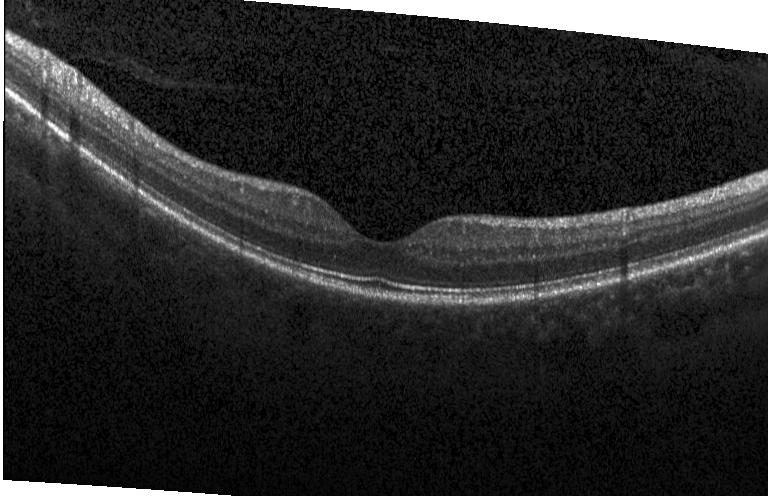

SD-OCT. Retinal OCT cross-section — Impression: no choroidal neovascularization, diabetic macular edema, or drusen.